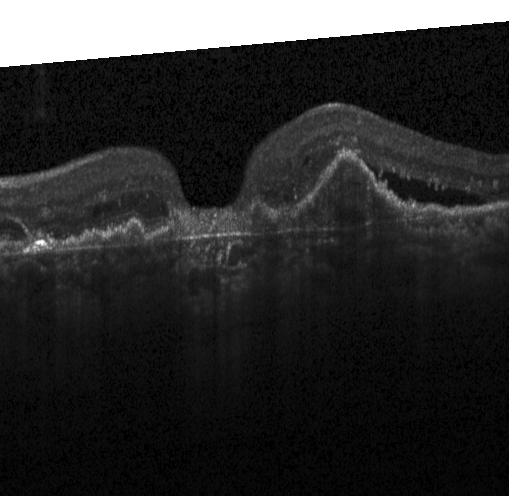 Finding: CNV.